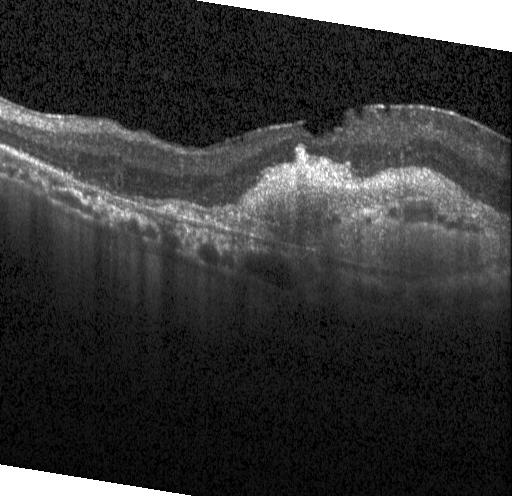 OCT line scan. Heidelberg Spectralis
Impression: choroidal neovascularization.